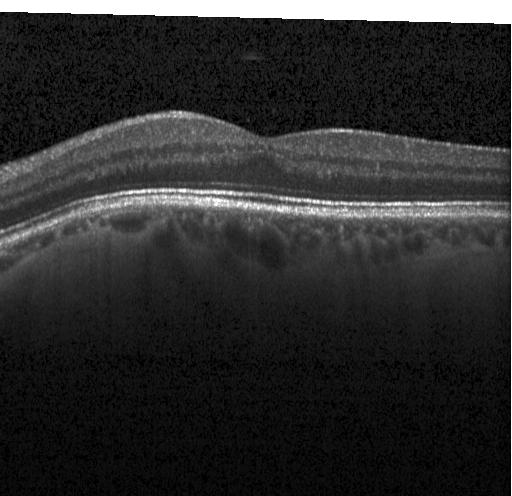

Retinal OCT B-scan · centered on the fovea
OCT finding: no CNV, no DME, and no drusen.